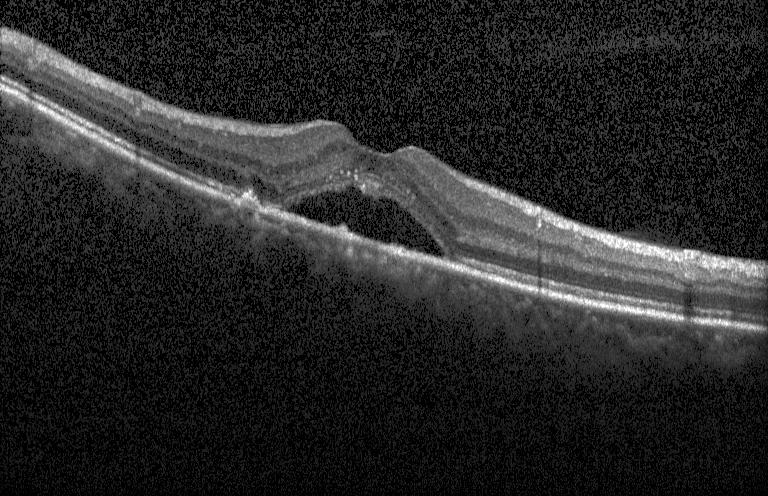 A choroidal neovascular membrane.